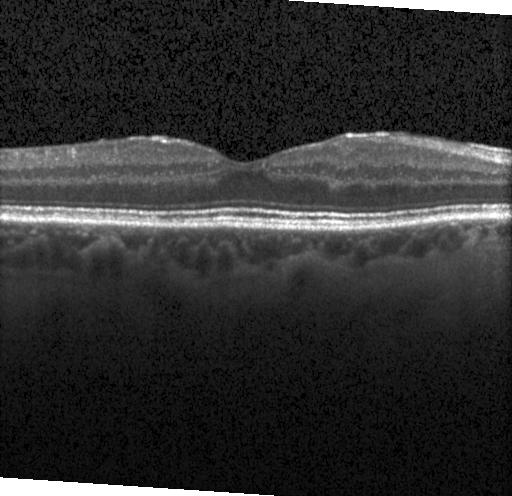 Centered on the fovea; spectral-domain OCT; Heidelberg Spectralis; retinal OCT B-scan — The scan shows no evidence of choroidal neovascularization, diabetic macular edema, or drusen.